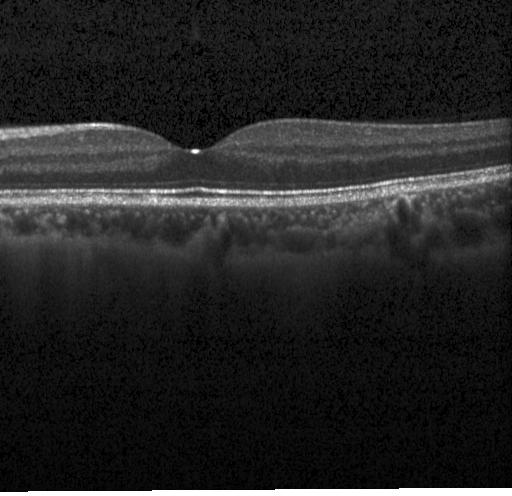 Spectral-domain OCT B-scan: no choroidal neovascularization, no diabetic macular edema, and no drusen.